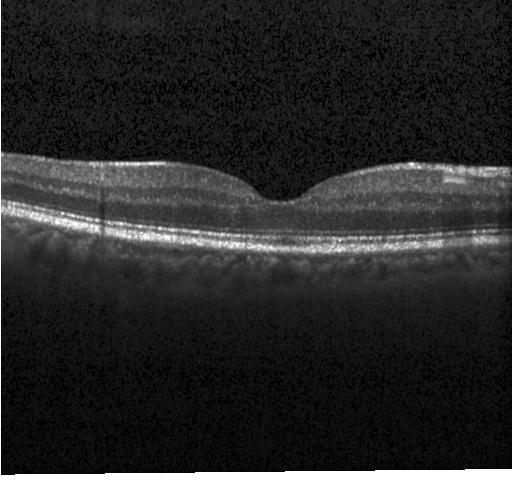
Spectral-domain OCT. Retinal OCT cross-section. Acquired on a Heidelberg Spectralis. Finding: no evidence of choroidal neovascularization, diabetic macular edema, or drusen.